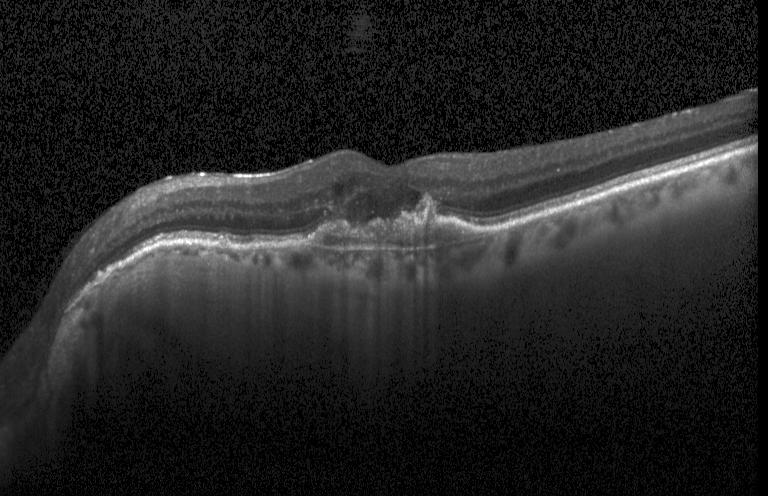
Horizontal scan through the fovea. OCT B-scan
Finding: a choroidal neovascular membrane.